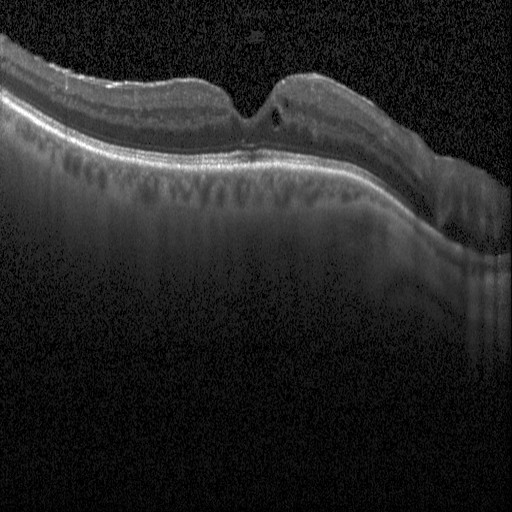

Finding: diabetic macular edema.